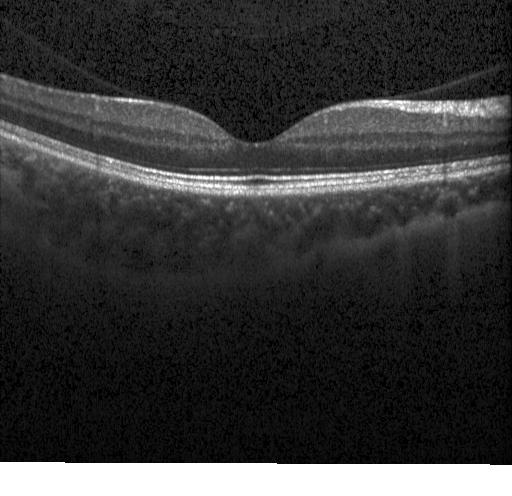
Spectral-domain optical coherence tomography. OCT B-scan. Macular OCT: no evidence of choroidal neovascularization, diabetic macular edema, or drusen.